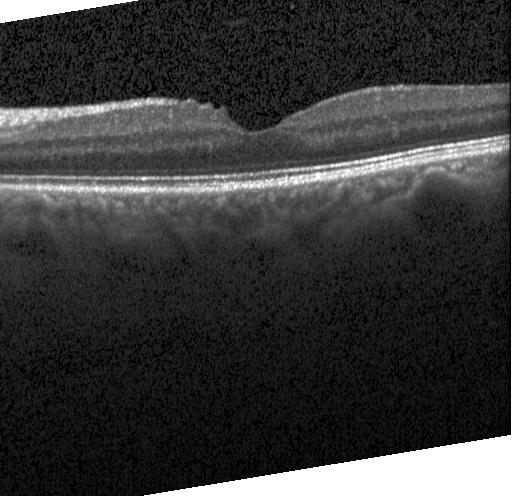 Optical coherence tomography scan · instrument: Heidelberg Spectralis · centered on the fovea. Diagnosis: no evidence of CNV, DME, or drusen.